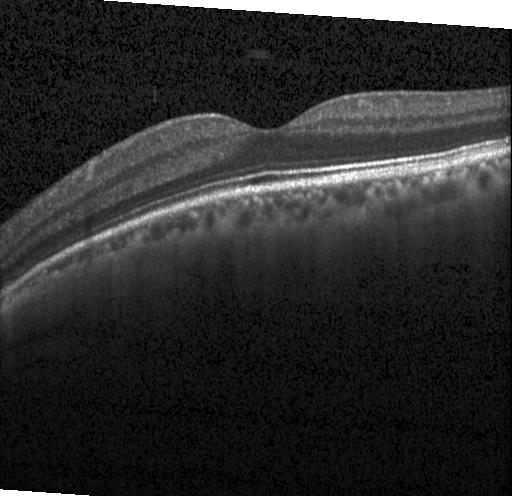

Retinal OCT cross-section showing no CNV, no DME, and no drusen.